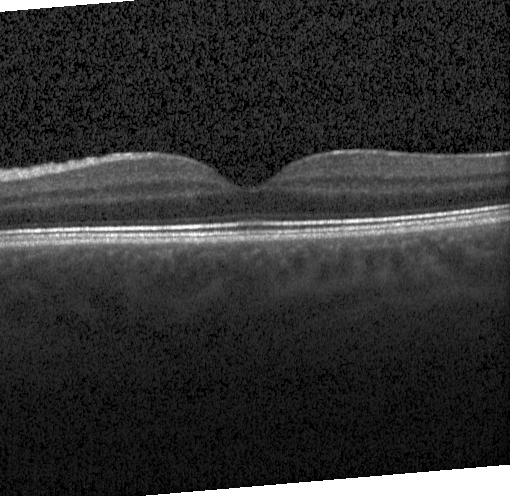

Retinal OCT B-scan.
Neither choroidal neovascularization, diabetic macular edema, nor drusen.